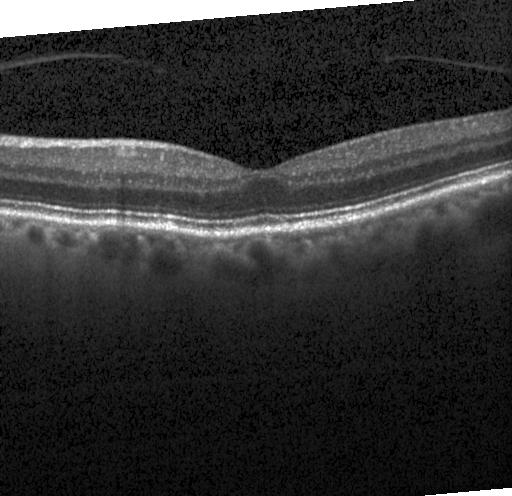 Retinal OCT B-scan — The scan shows no evidence of choroidal neovascularization, diabetic macular edema, or drusen.